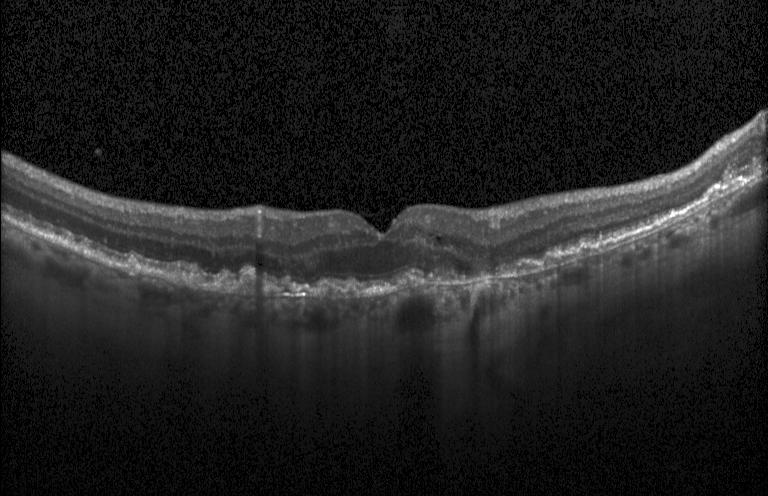

Heidelberg Spectralis. Fovea-centered. Optical coherence tomography scan. Spectral-domain optical coherence tomography. Finding: a choroidal neovascular membrane.